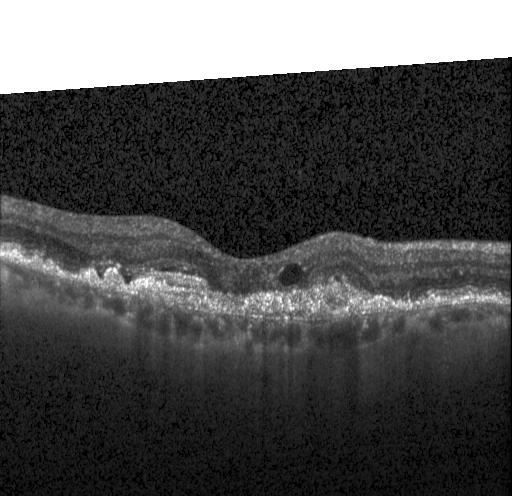
Finding: a choroidal neovascular membrane.